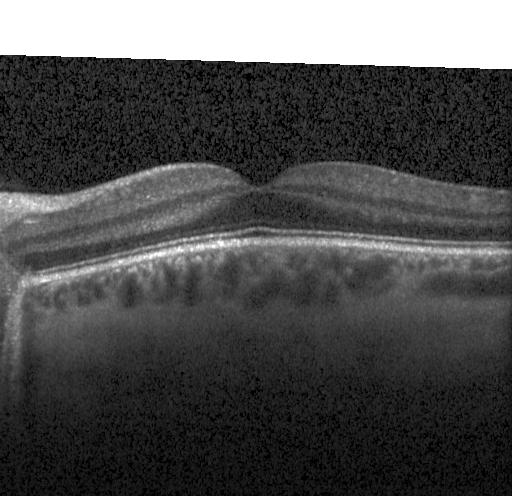

Impression: no choroidal neovascularization, no diabetic macular edema, and no drusen.